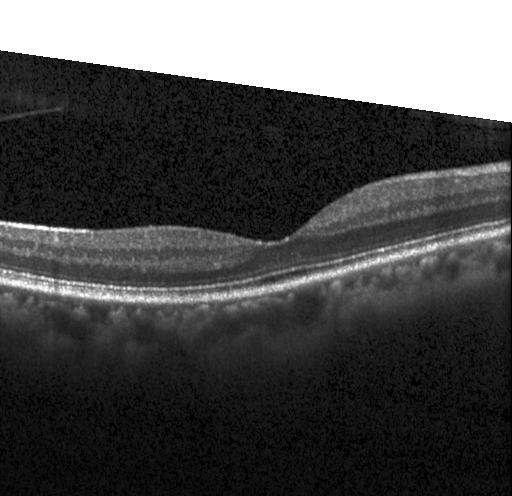 Retinal OCT cross-section. OCT finding: no choroidal neovascularization, no diabetic macular edema, and no drusen.